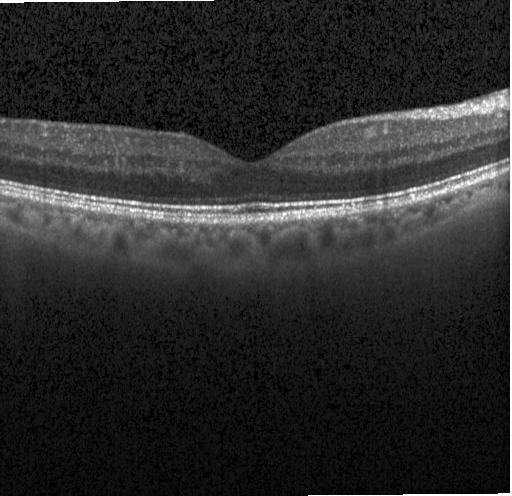

OCT scan showing no evidence of choroidal neovascularization, diabetic macular edema, or drusen.